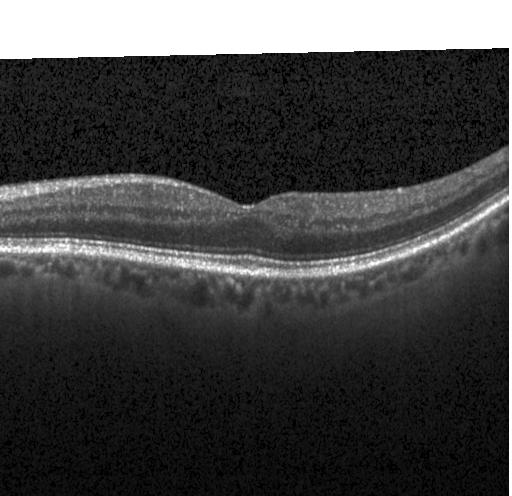
Optical coherence tomography B-scan. Acquired on a Heidelberg Spectralis — Macular OCT: no evidence of choroidal neovascularization, diabetic macular edema, or drusen.